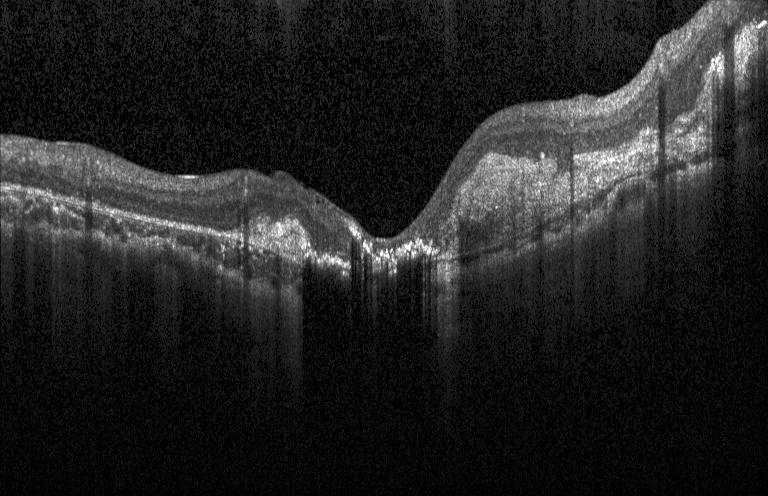

Finding: choroidal neovascularization.